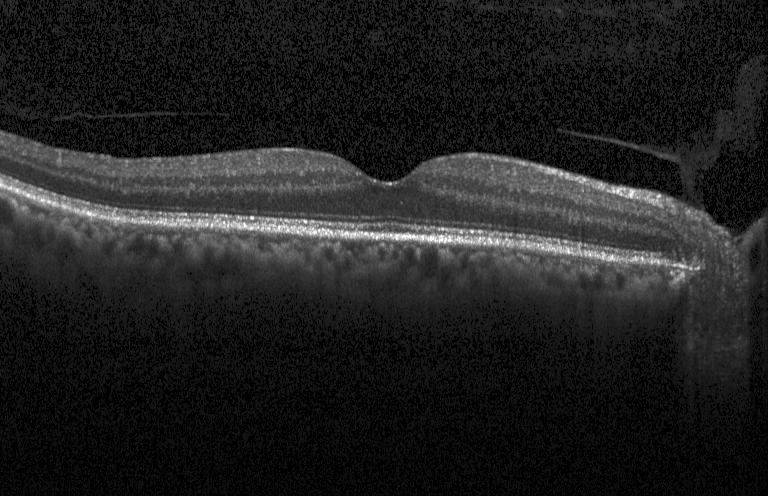

Retinal OCT cross-section showing no evidence of CNV, DME, or drusen.